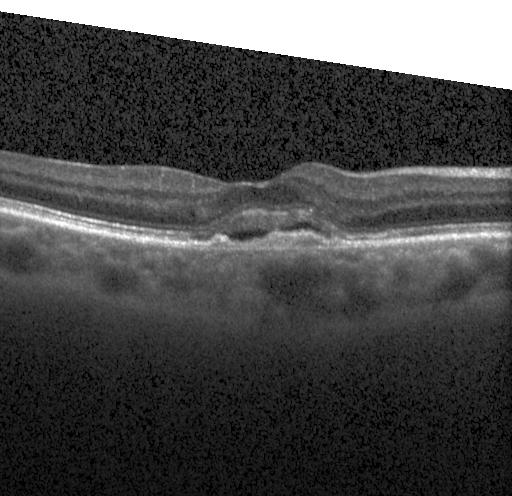 Retinal OCT cross-section showing a choroidal neovascular membrane.